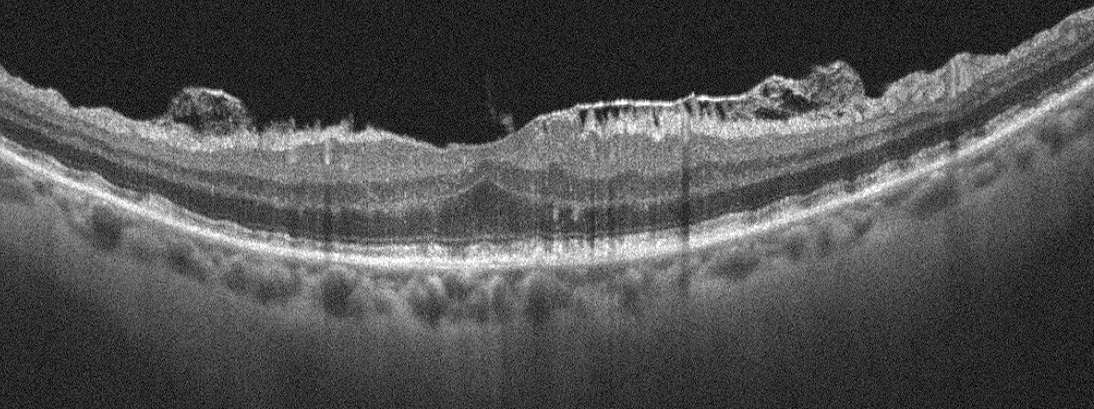
Retinal OCT B-scan — Diagnosis: ERM.